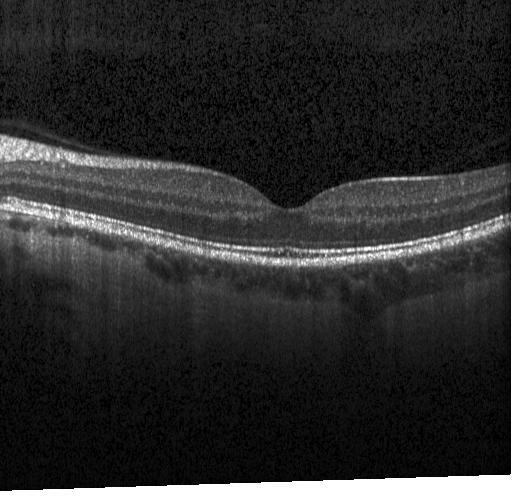

Finding: no choroidal neovascularization, diabetic macular edema, or drusen.